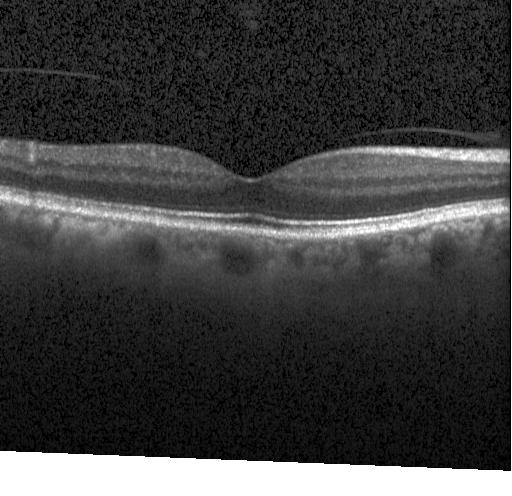 Instrument: Heidelberg Spectralis; optical coherence tomography scan; spectral-domain optical coherence tomography; horizontal scan through the fovea. OCT finding: no choroidal neovascularization, no diabetic macular edema, and no drusen.